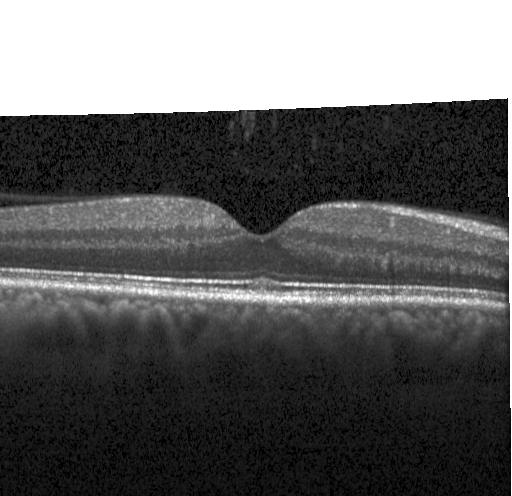
OCT line scan. Finding: no CNV, no DME, and no drusen.